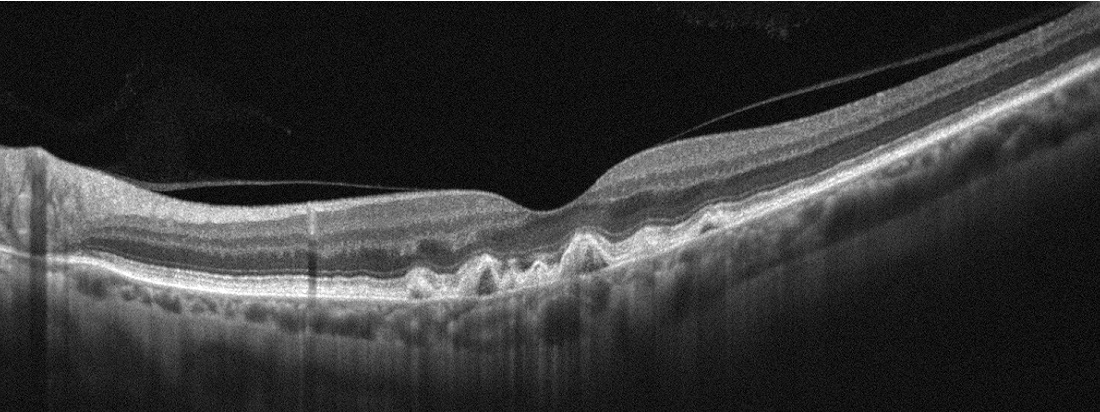
Instrument: Optovue Avanti RTVue XR, retinal OCT B-scan.
Assessment: age-related macular degeneration (AMD).